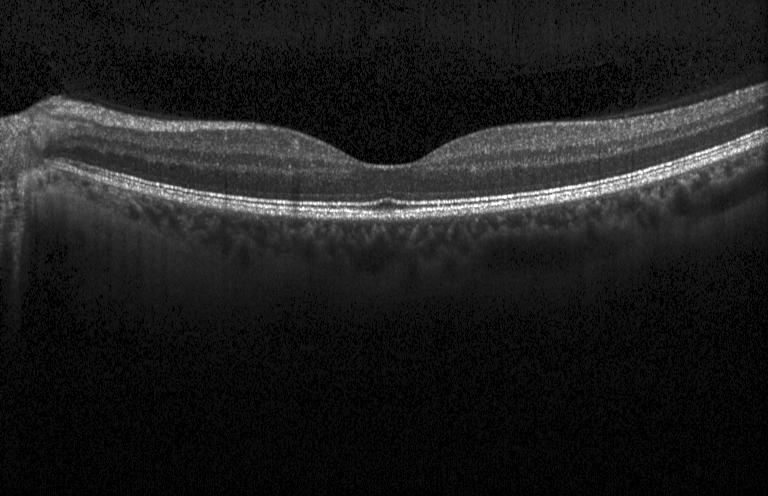

OCT line scan. Heidelberg Spectralis. SD-OCT. Fovea-centered
Finding: no CNV, DME, or drusen.